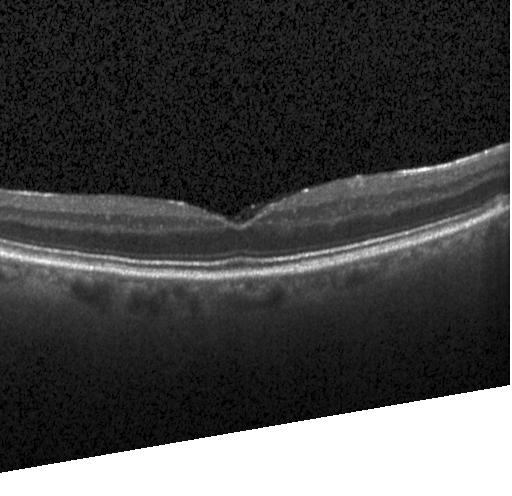
Fovea-centered. OCT line scan. Instrument: Heidelberg Spectralis. SD-OCT
OCT finding: neither choroidal neovascularization, diabetic macular edema, nor drusen.